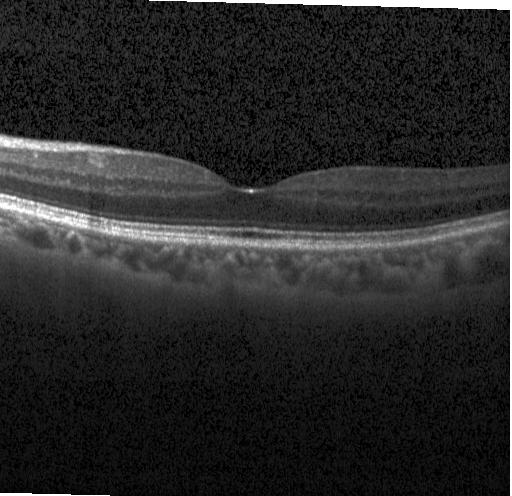

Macular OCT demonstrating no choroidal neovascularization, no diabetic macular edema, and no drusen.